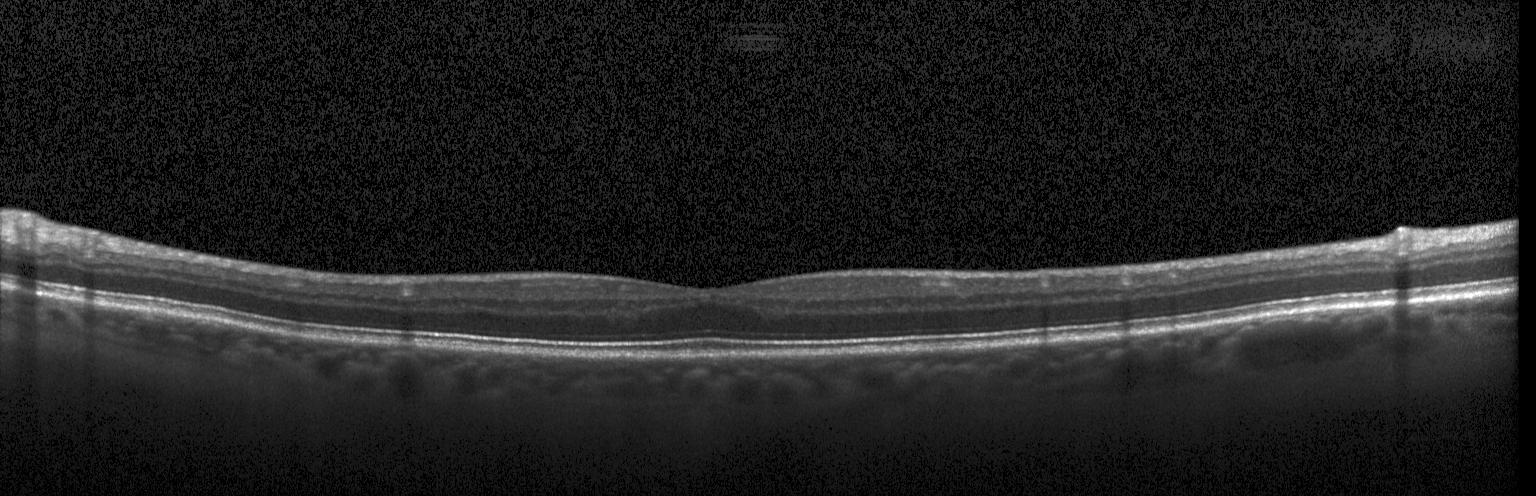

The scan shows no evidence of choroidal neovascularization, diabetic macular edema, or drusen.